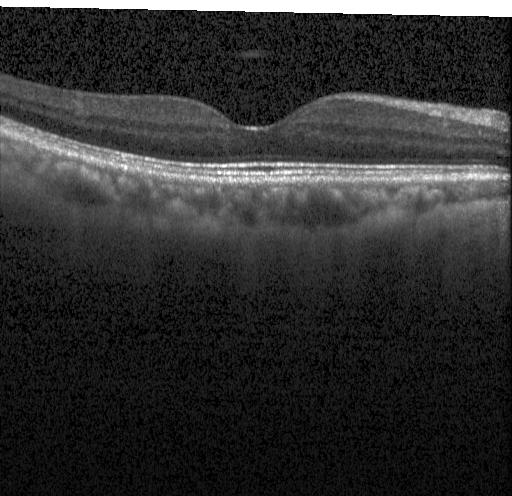 Assessment: no choroidal neovascularization, no diabetic macular edema, and no drusen.